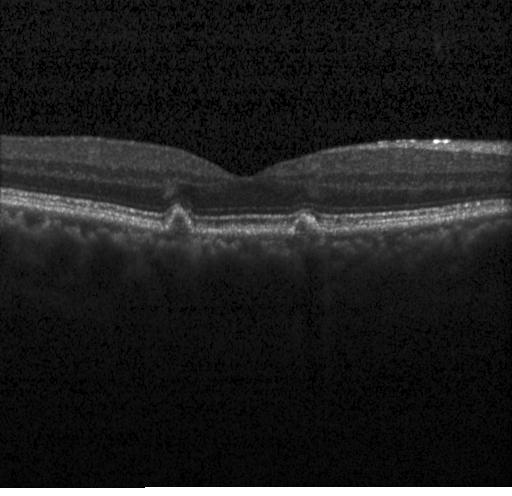
Assessment: drusen.